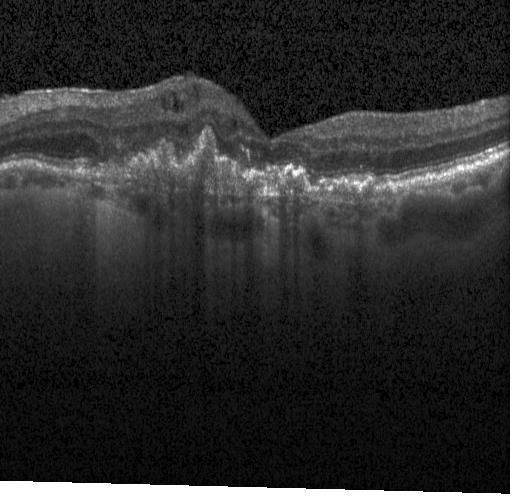 OCT finding: a choroidal neovascular membrane.